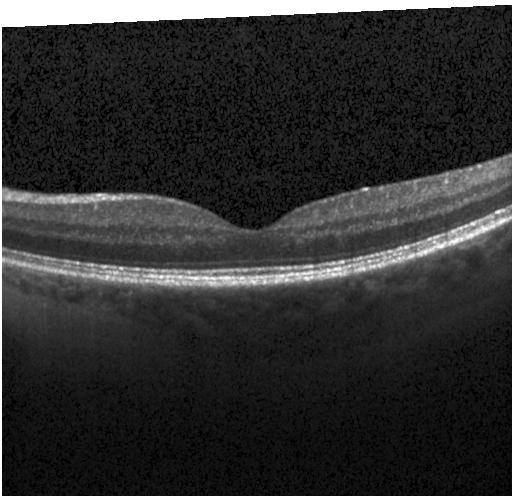
Through the macula; Heidelberg Spectralis OCT system; OCT line scan.
Assessment: neither choroidal neovascularization, diabetic macular edema, nor drusen.